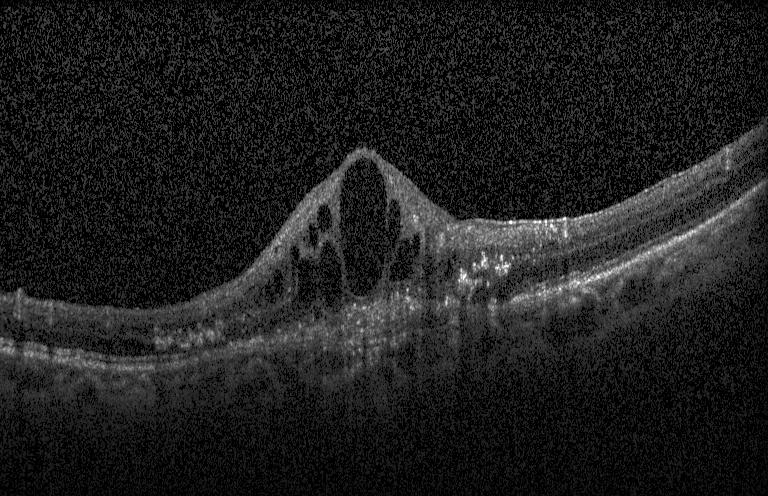
Macular scan; Heidelberg Spectralis; spectral-domain optical coherence tomography; retinal OCT B-scan — Macular OCT: choroidal neovascularization (CNV).